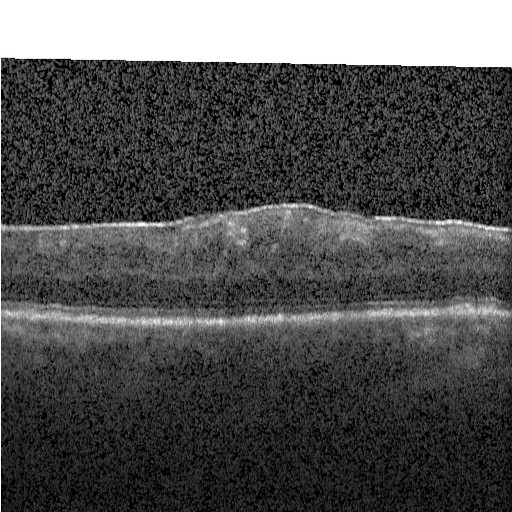

This B-scan demonstrates diabetic macular edema.